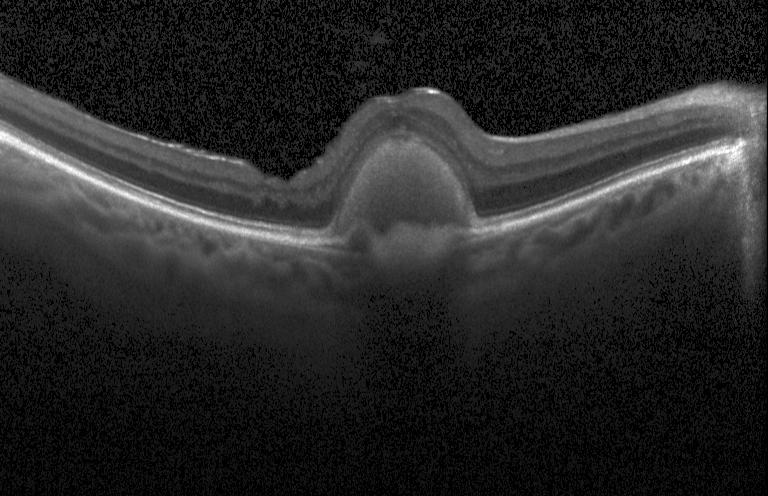 Finding: a choroidal neovascular membrane.